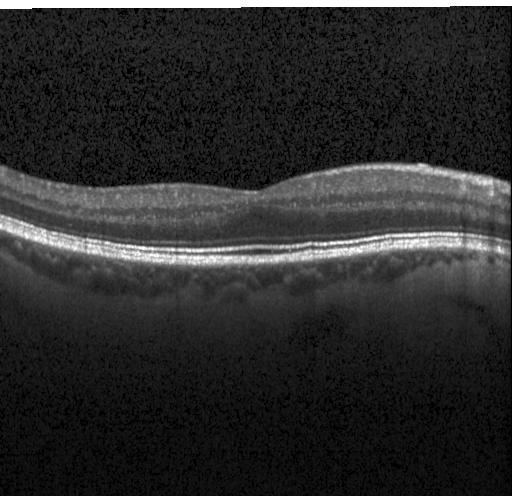
The scan shows neither choroidal neovascularization, diabetic macular edema, nor drusen.